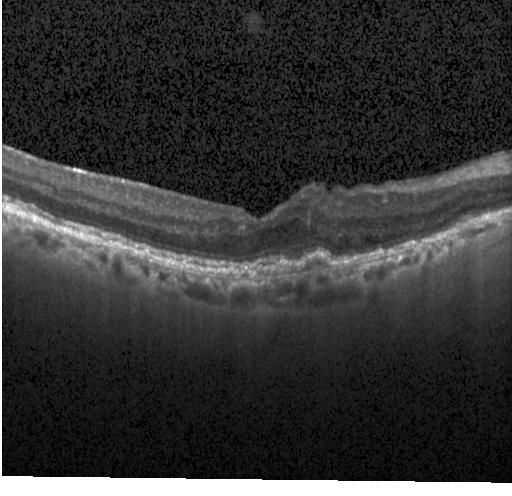 Fovea-centered. Retinal OCT B-scan. Spectral-domain optical coherence tomography. Impression: a choroidal neovascular membrane.